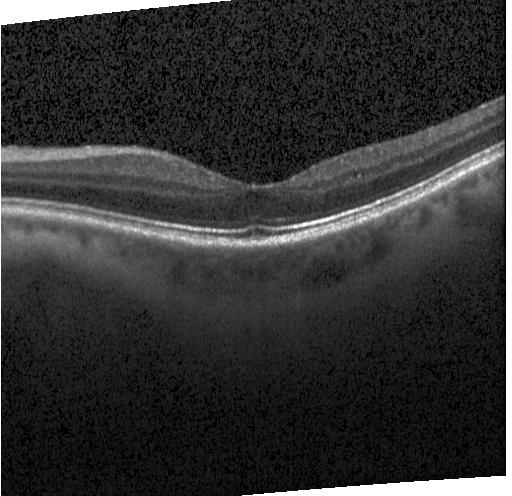
Heidelberg Spectralis; OCT line scan; SD-OCT; fovea-centered. Finding: no CNV, no DME, and no drusen.